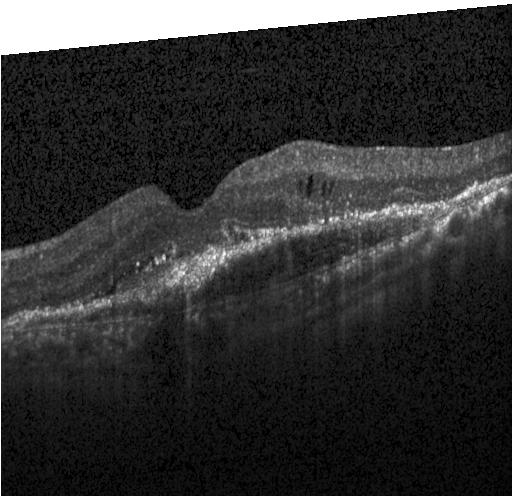

OCT scan showing choroidal neovascularization.